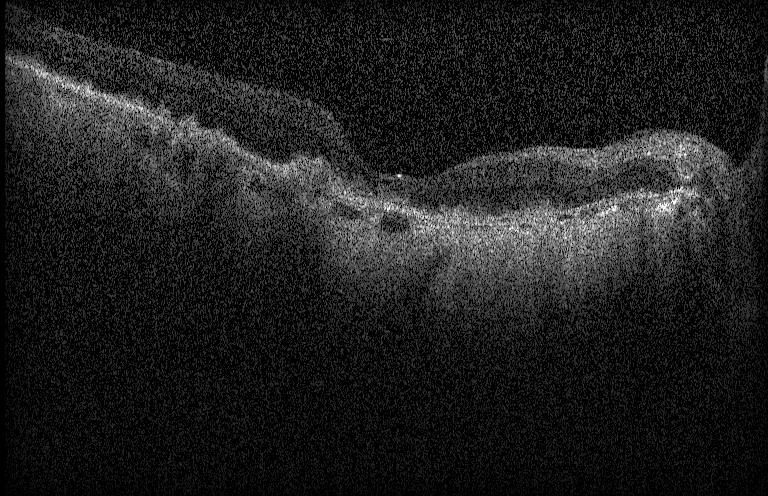 Heidelberg Spectralis; fovea-centered; spectral-domain optical coherence tomography; OCT line scan.
Macular OCT: a choroidal neovascular membrane.